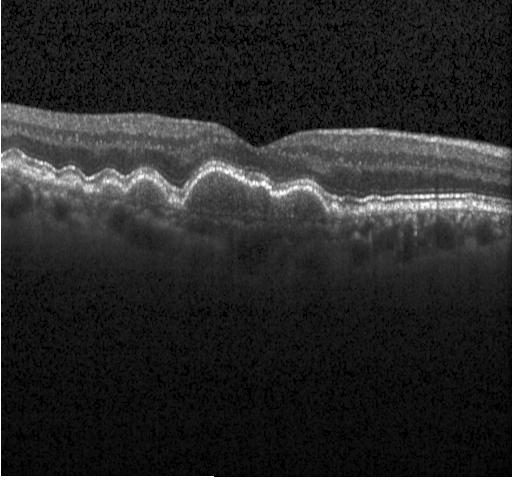
Retinal OCT cross-section showing sub-RPE drusenoid deposits.